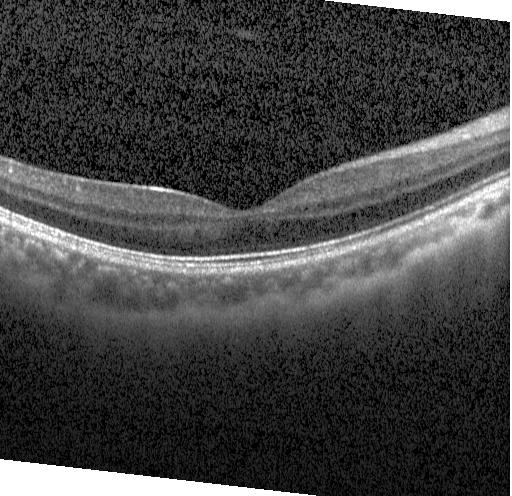

Diagnosis: no CNV, no DME, and no drusen.